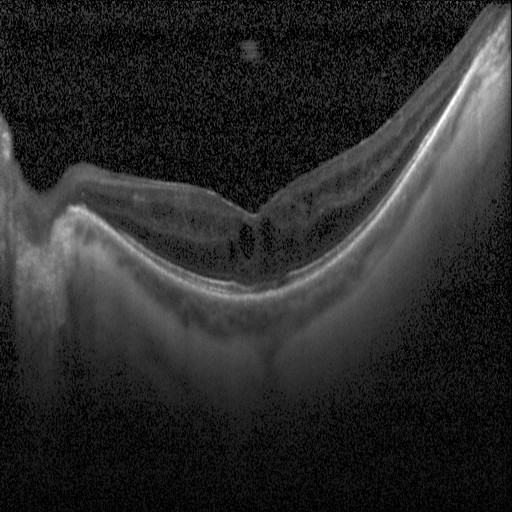
SD-OCT; OCT line scan; centered on the fovea — The scan shows diabetic macular edema (DME).